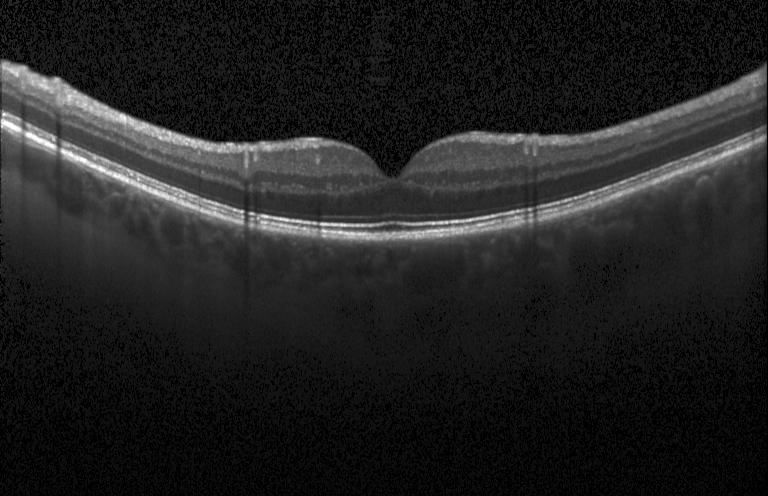

OCT finding: no evidence of choroidal neovascularization, diabetic macular edema, or drusen.